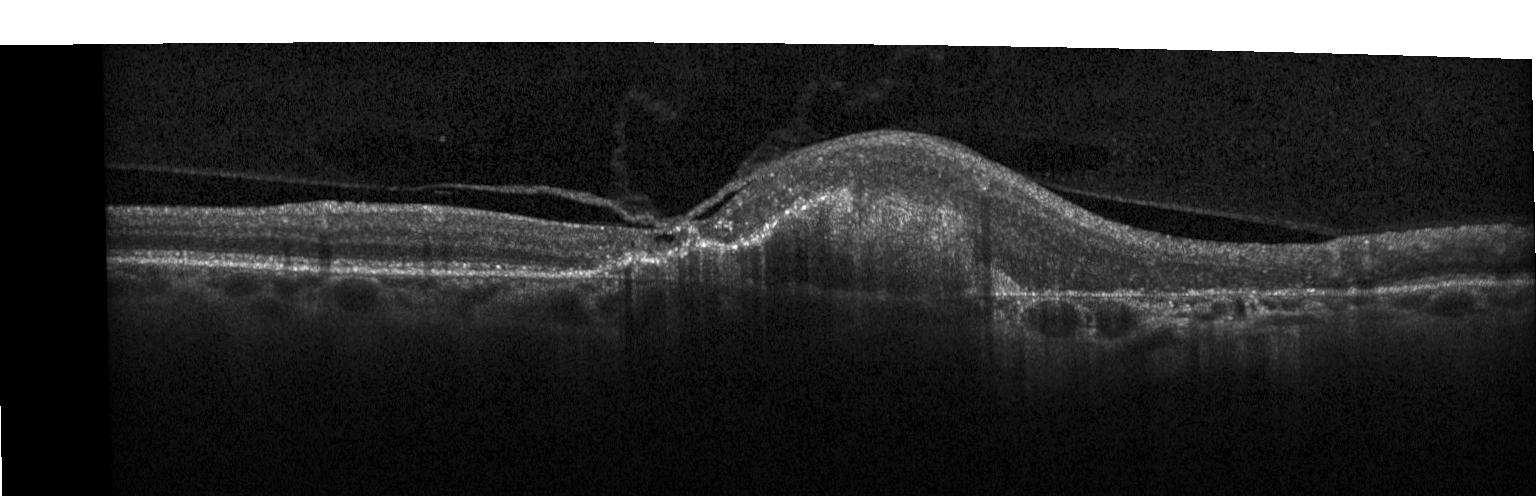

OCT line scan; spectral-domain OCT. This B-scan demonstrates choroidal neovascularization.